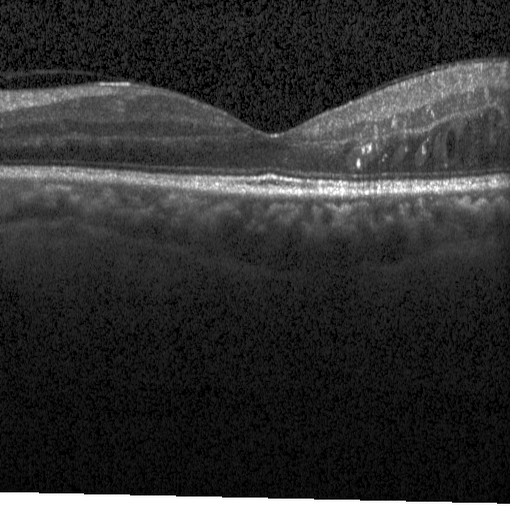 Heidelberg Spectralis · retinal OCT B-scan.
Finding: DME.